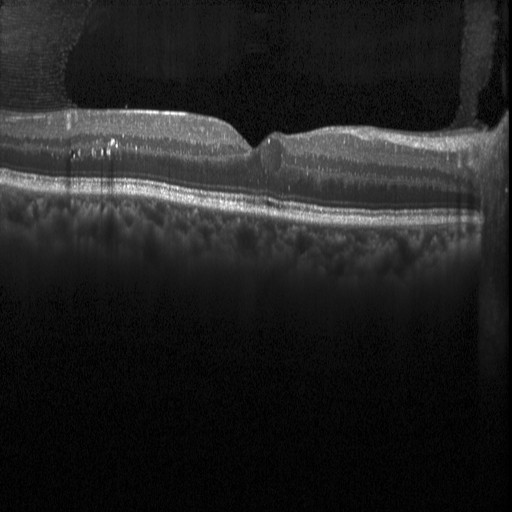 Retinal OCT B-scan. Finding: DME.